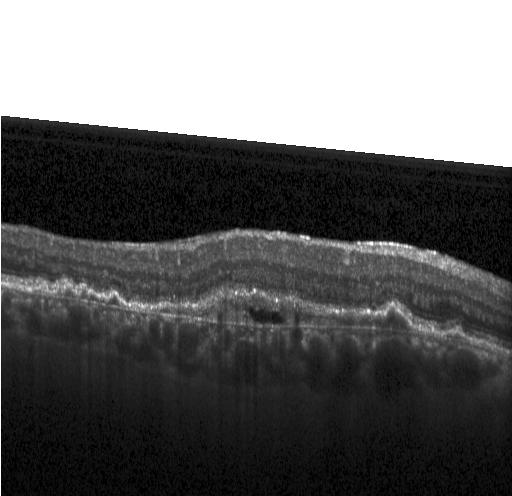
Optical coherence tomography scan.
Dx: a choroidal neovascular membrane.